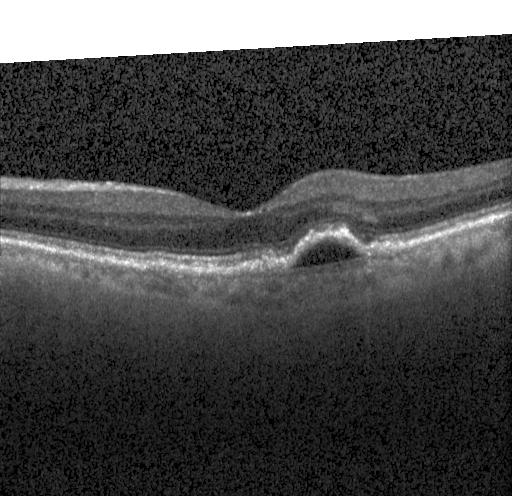

Optical coherence tomography scan. Heidelberg Spectralis. Spectral-domain optical coherence tomography — Macular OCT: a choroidal neovascular membrane.